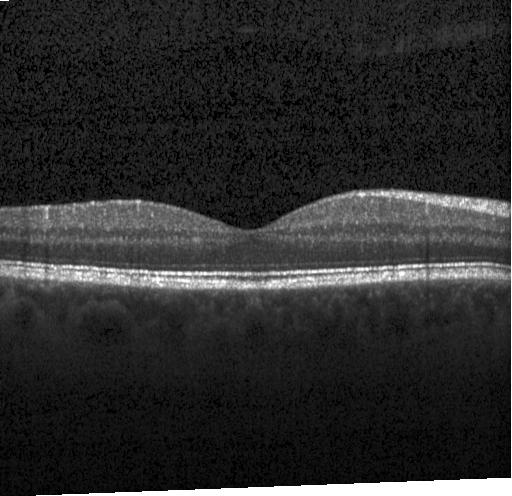 Optical coherence tomography scan; Heidelberg Spectralis. Diagnosis: neither CNV, DME, nor drusen.